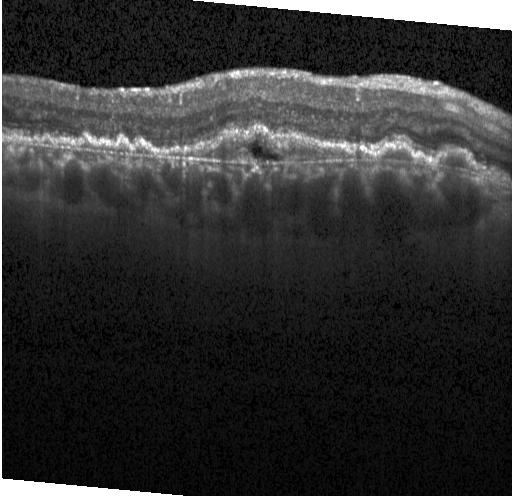

Optical coherence tomography scan — Diagnosis: a choroidal neovascular membrane.